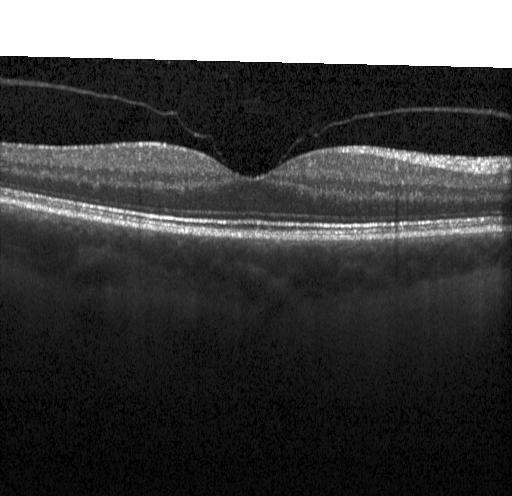

Diagnosis: no evidence of CNV, DME, or drusen.